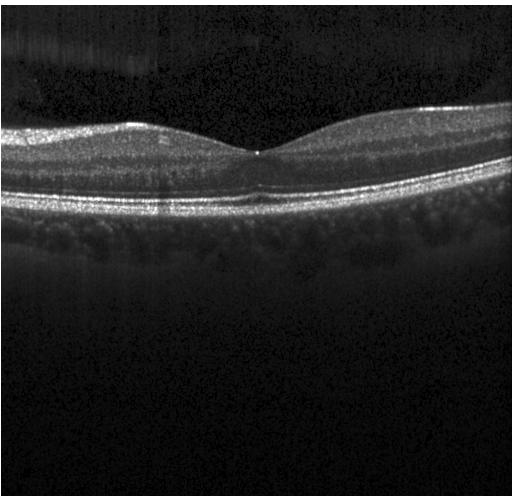
Optical coherence tomography B-scan · Heidelberg Spectralis OCT system · centered on the fovea. No choroidal neovascularization, no diabetic macular edema, and no drusen.